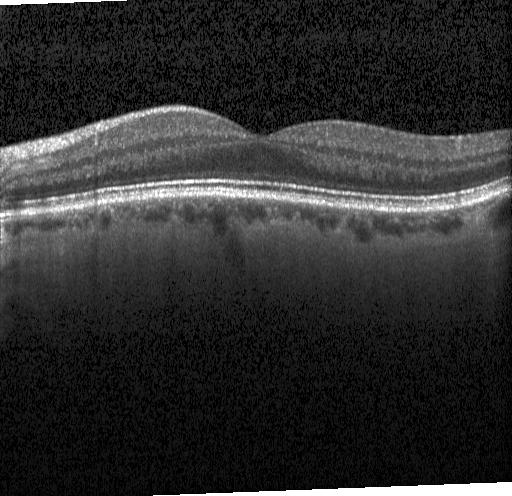

OCT line scan. Fovea-centered. The scan shows no choroidal neovascularization, diabetic macular edema, or drusen.